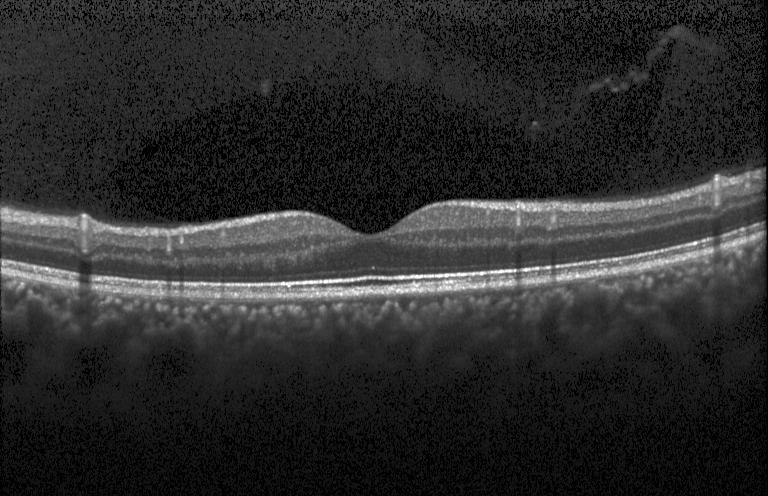

SD-OCT; instrument: Heidelberg Spectralis; optical coherence tomography scan. OCT finding: neither CNV, DME, nor drusen.